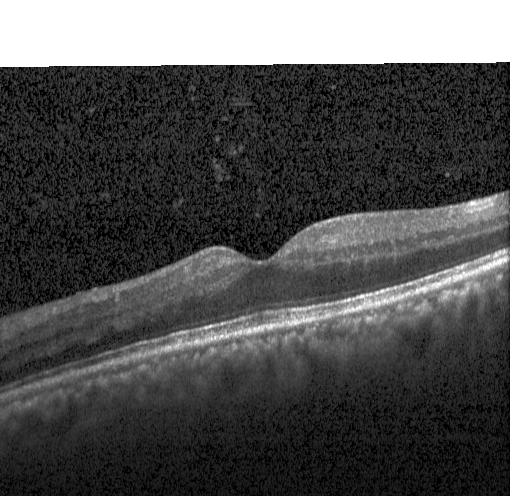

Optical coherence tomography scan, Heidelberg Spectralis OCT system, SD-OCT — Finding: neither choroidal neovascularization, diabetic macular edema, nor drusen.